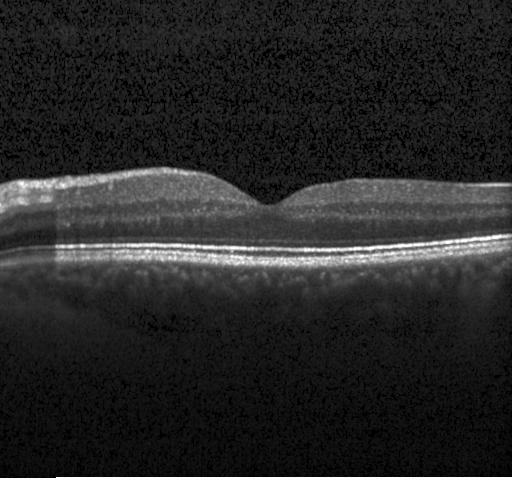
Spectral-domain OCT. OCT line scan
Assessment: neither choroidal neovascularization, diabetic macular edema, nor drusen.